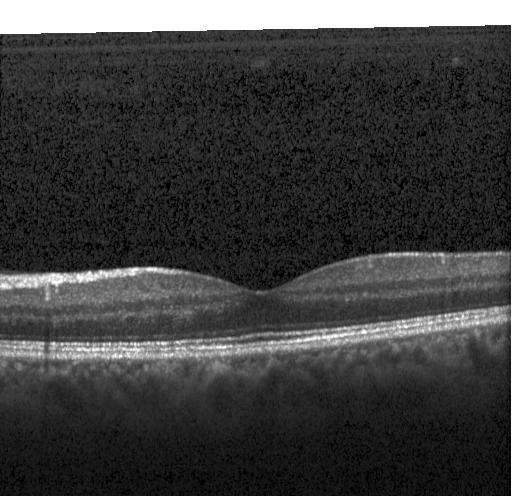
SD-OCT · horizontal scan through the fovea · optical coherence tomography scan · Heidelberg Spectralis OCT system — No choroidal neovascularization, diabetic macular edema, or drusen.